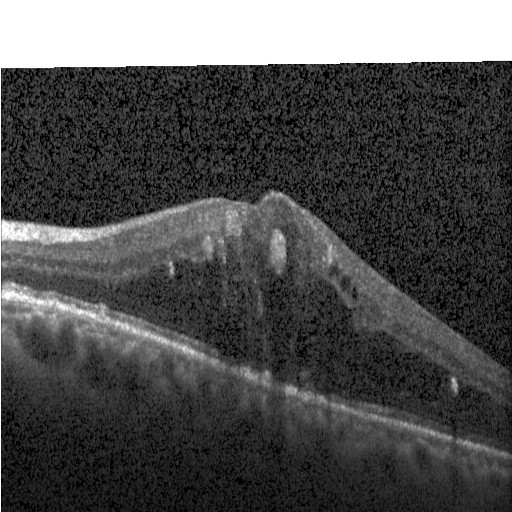 Horizontal scan through the fovea; acquired on a Heidelberg Spectralis; optical coherence tomography scan; spectral-domain OCT — OCT finding: diabetic macular edema (DME).